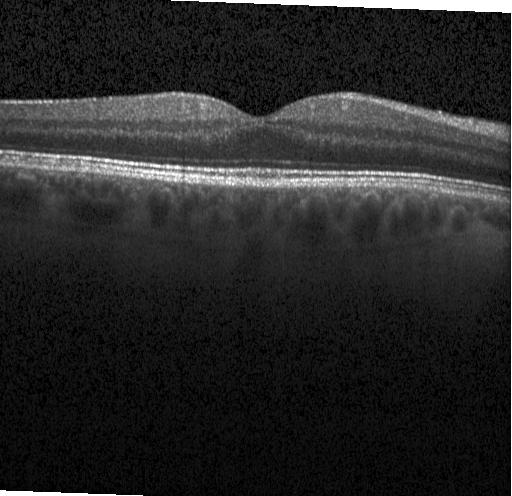
Neither choroidal neovascularization, diabetic macular edema, nor drusen.